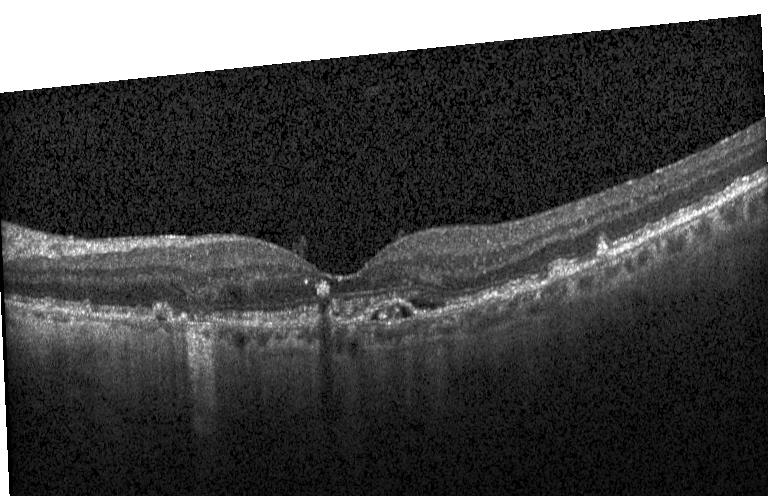 OCT scan showing choroidal neovascularization (CNV).